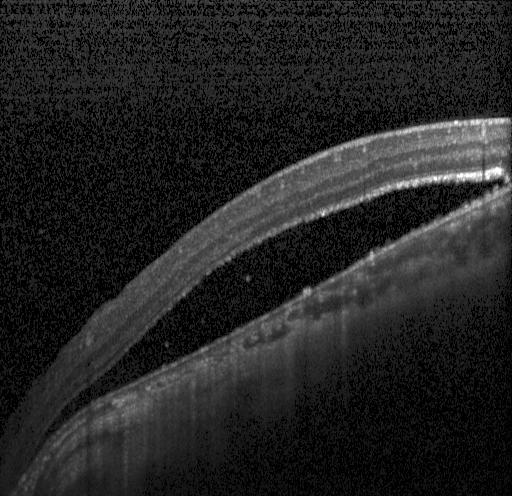 Diagnosis: CNV.